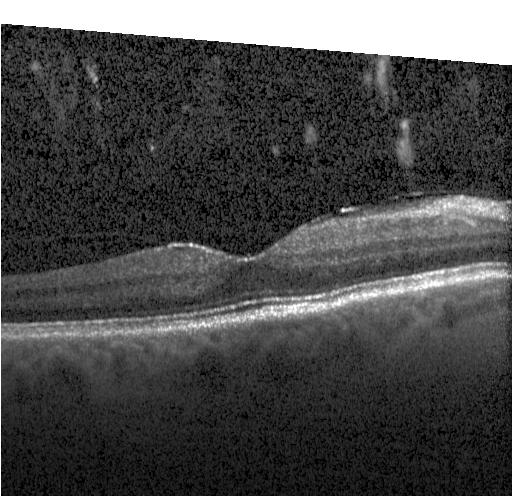
OCT B-scan — Neither choroidal neovascularization, diabetic macular edema, nor drusen.